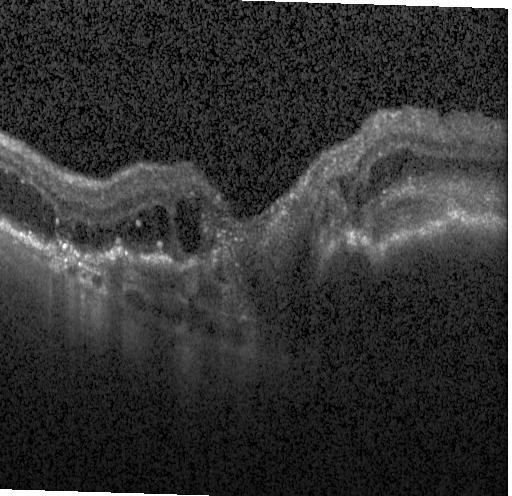

OCT B-scan showing a choroidal neovascular membrane.